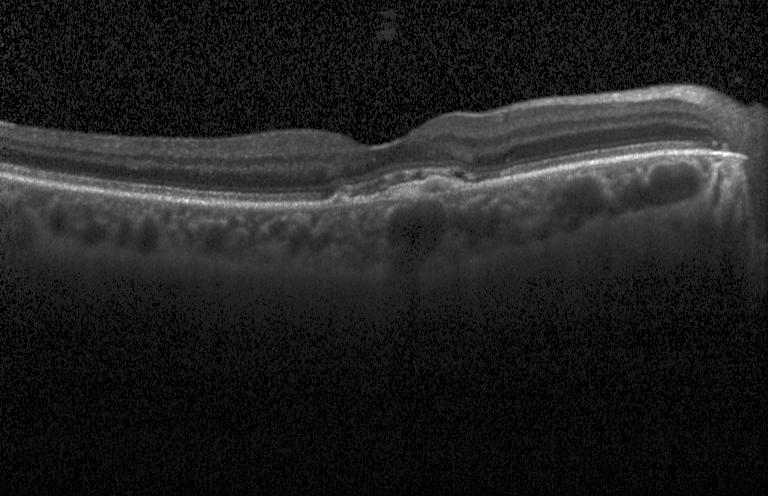
OCT B-scan — Macular OCT: a choroidal neovascular membrane.